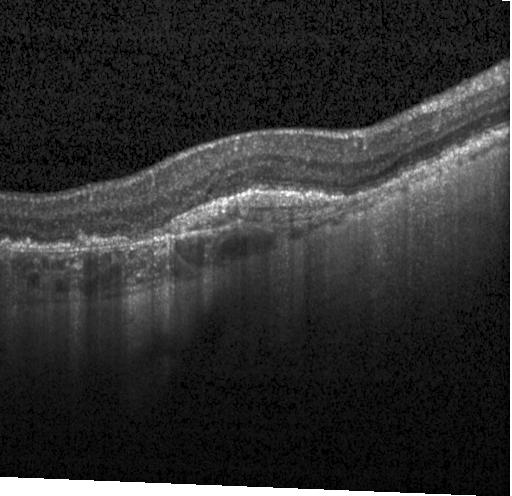
Retinal OCT B-scan
Assessment: choroidal neovascularization.